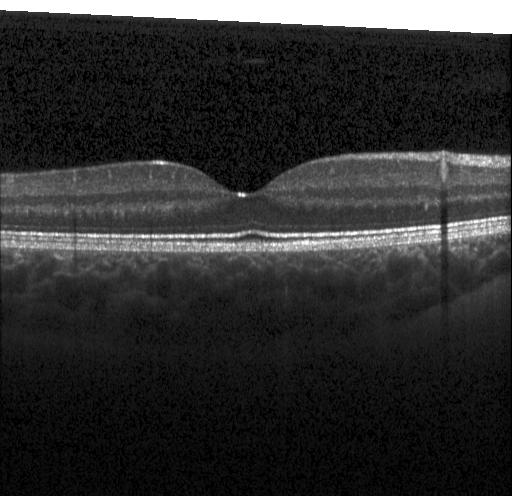 Retinal OCT B-scan, SD-OCT, acquired on a Heidelberg Spectralis, macular scan
Impression: neither choroidal neovascularization, diabetic macular edema, nor drusen.